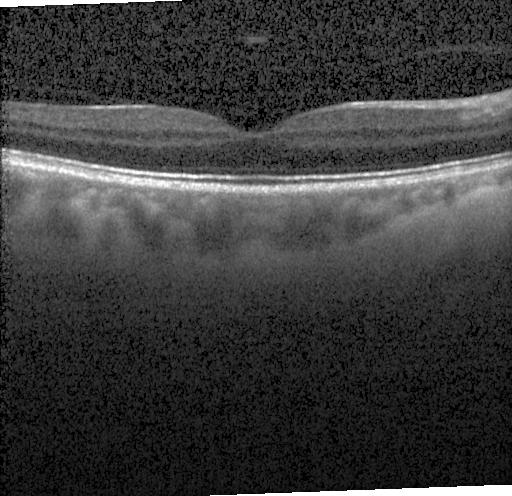 Retinal OCT cross-section · instrument: Heidelberg Spectralis
Dx: neither choroidal neovascularization, diabetic macular edema, nor drusen.